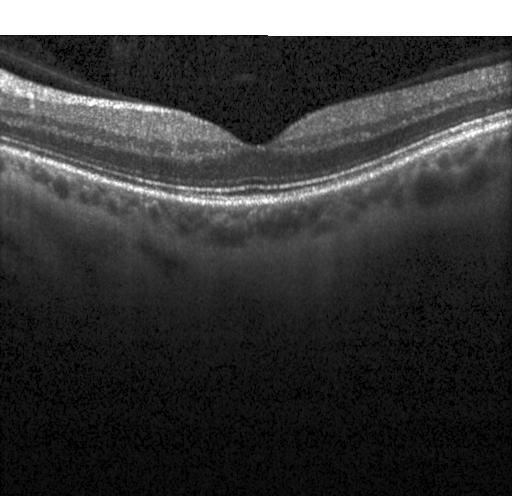 Spectral-domain OCT. Through the macula. OCT line scan — This B-scan demonstrates no choroidal neovascularization, diabetic macular edema, or drusen.